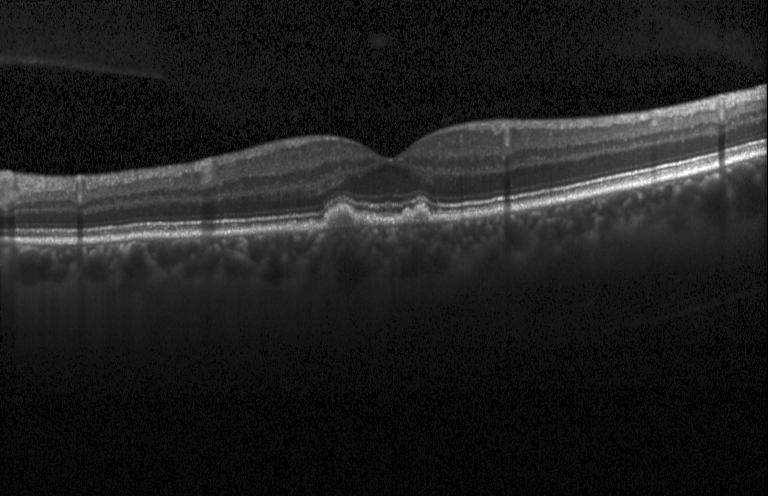 Dx: multiple drusen.